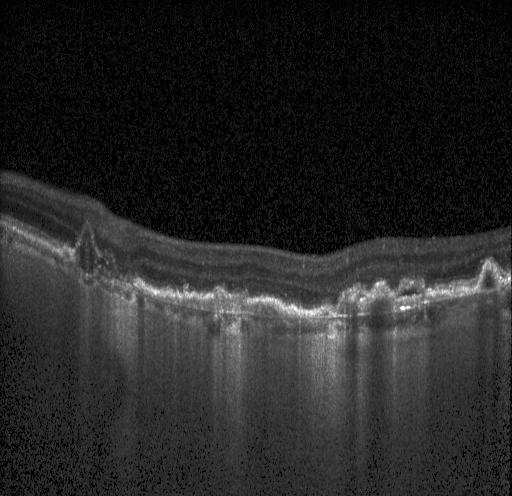 Retinal OCT cross-section — OCT finding: a choroidal neovascular membrane.